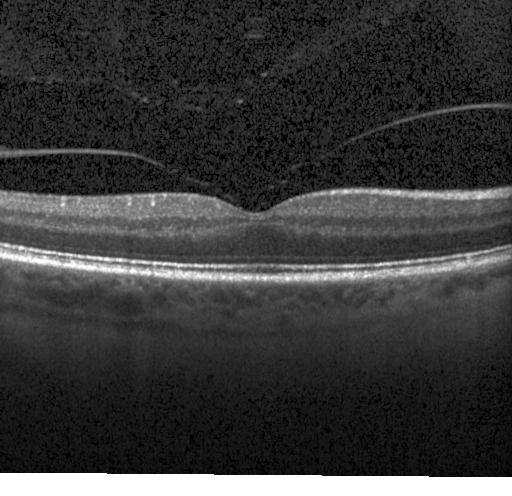

Heidelberg Spectralis, OCT line scan.
This B-scan demonstrates no CNV, DME, or drusen.